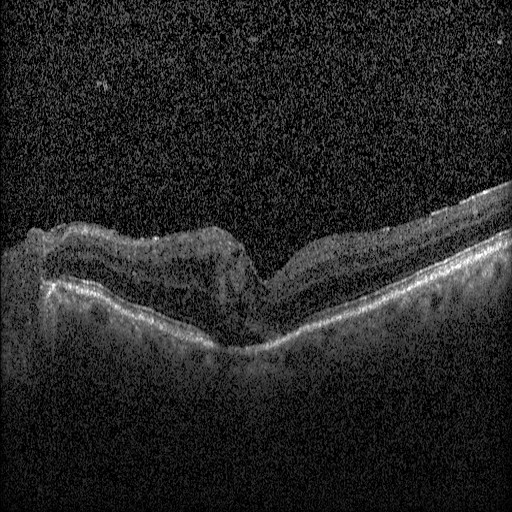 Centered on the fovea, OCT line scan, acquired on a Heidelberg Spectralis. This B-scan demonstrates DME.